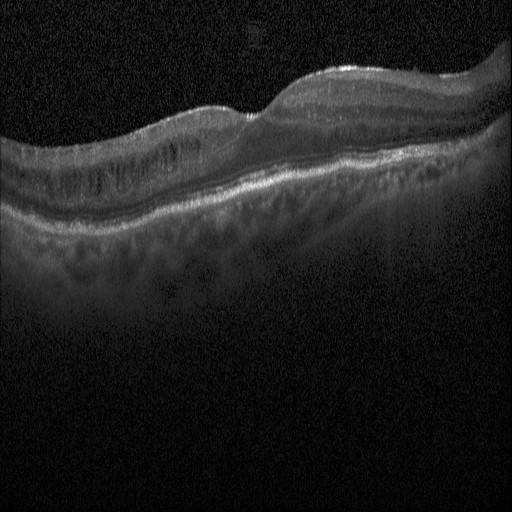 SD-OCT, optical coherence tomography scan. Impression: DME.